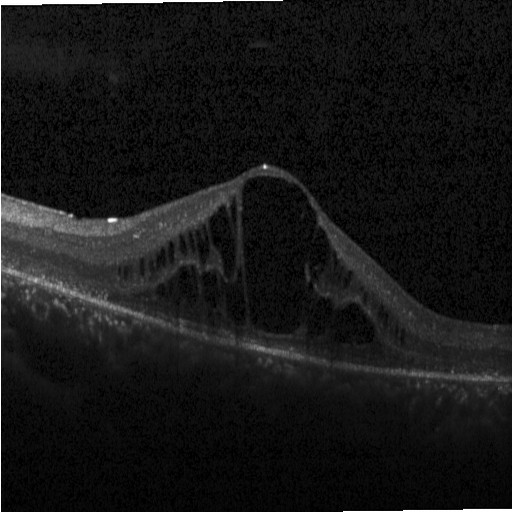 Macular OCT demonstrating diabetic macular edema (DME).